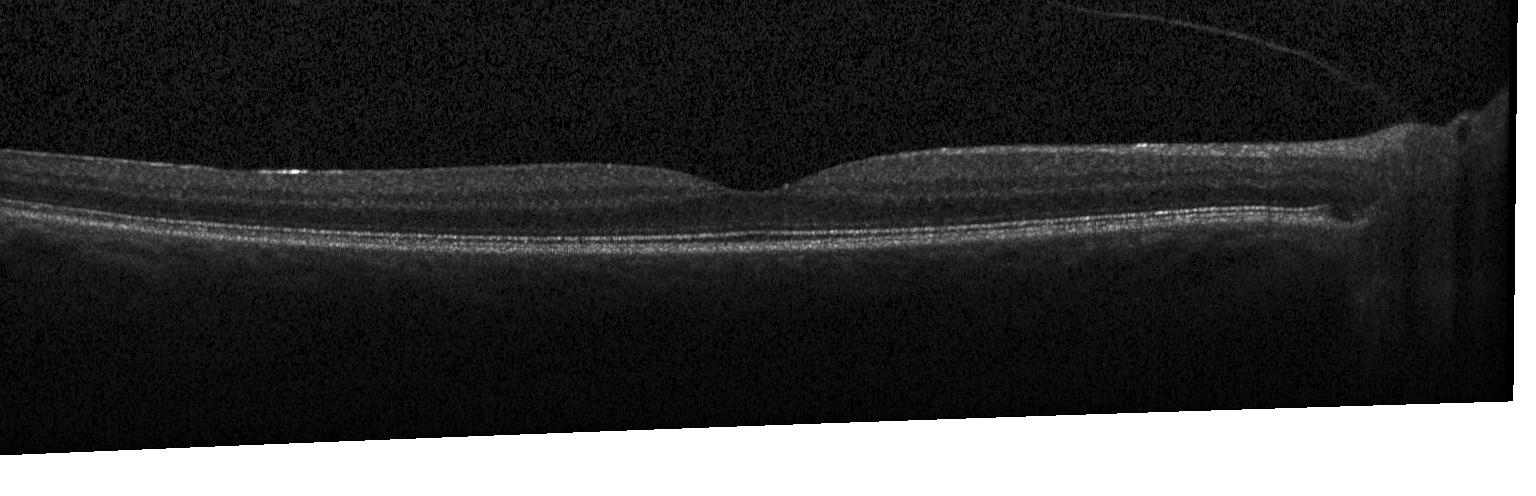
SD-OCT; retinal OCT cross-section — Assessment: no choroidal neovascularization, no diabetic macular edema, and no drusen.